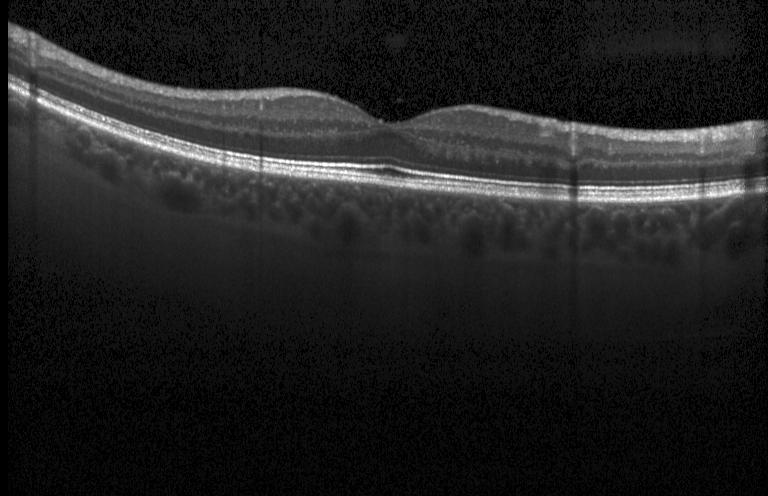
Retinal OCT B-scan.
No choroidal neovascularization, no diabetic macular edema, and no drusen.